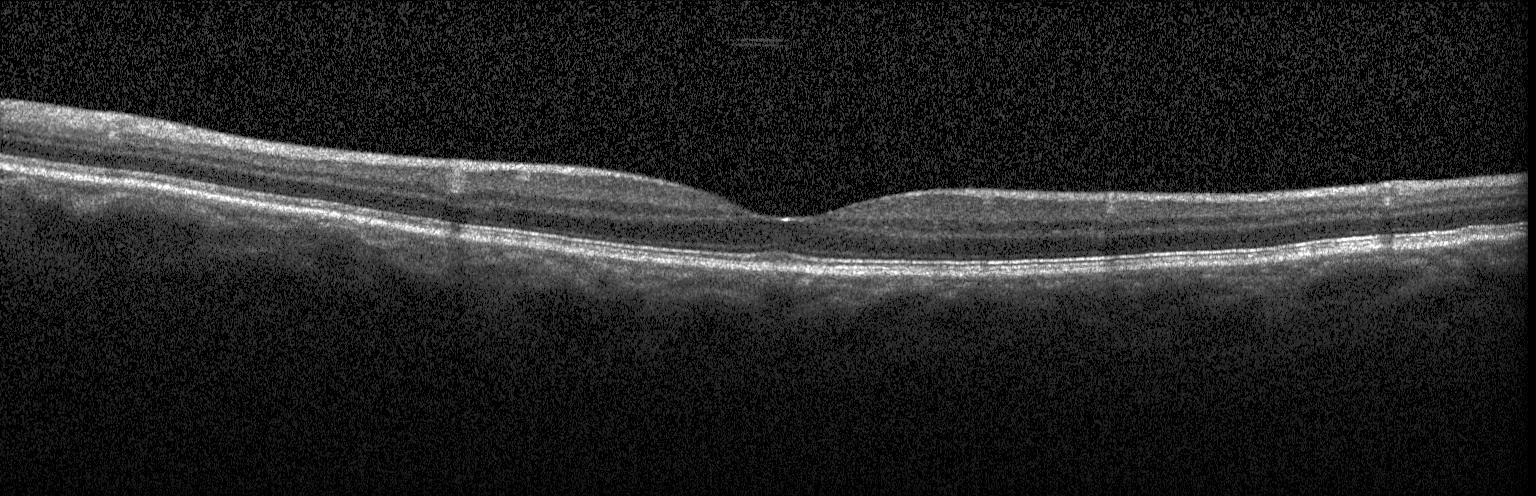

Heidelberg Spectralis OCT system, retinal OCT cross-section.
Diagnosis: no evidence of choroidal neovascularization, diabetic macular edema, or drusen.